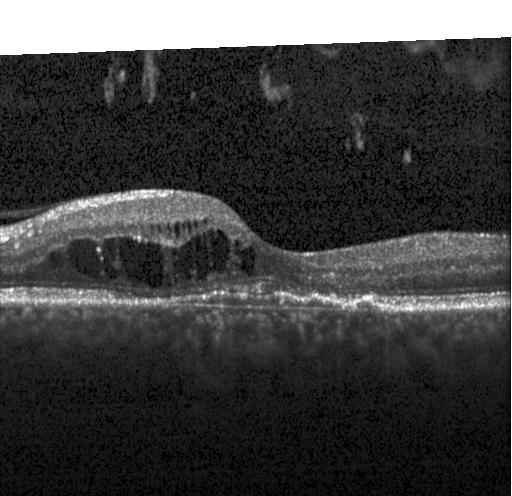

Retinal OCT B-scan, spectral-domain optical coherence tomography. Finding: choroidal neovascularization.